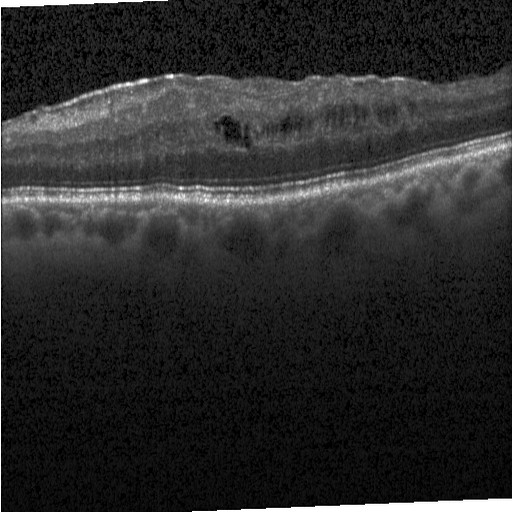
Fovea-centered; Heidelberg Spectralis OCT system; SD-OCT; OCT line scan
Macular OCT: diabetic macular edema.